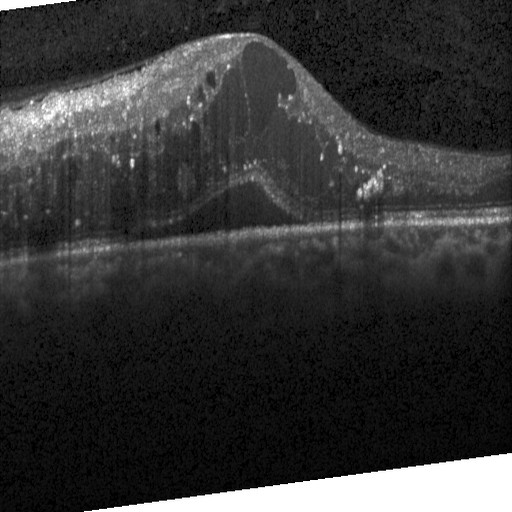

Finding: diabetic macular edema (DME).